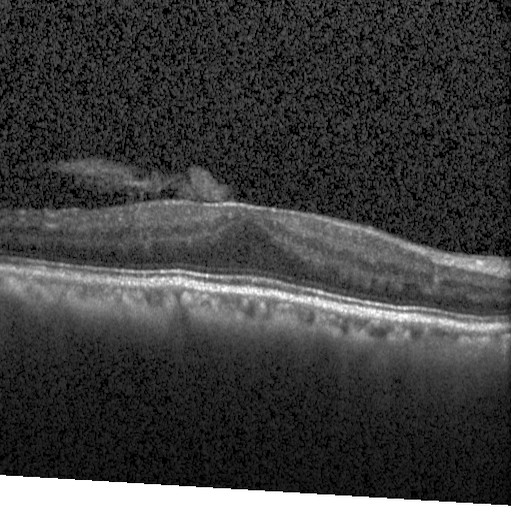
OCT line scan.
Impression: DME.